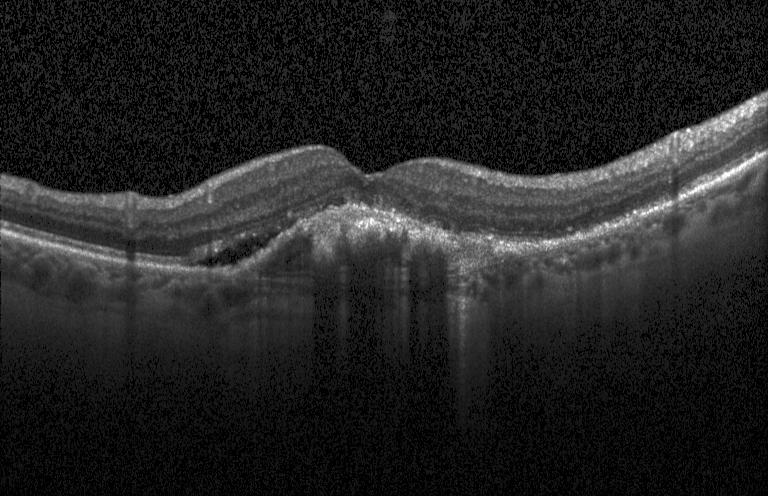 OCT B-scan. Finding: choroidal neovascularization.